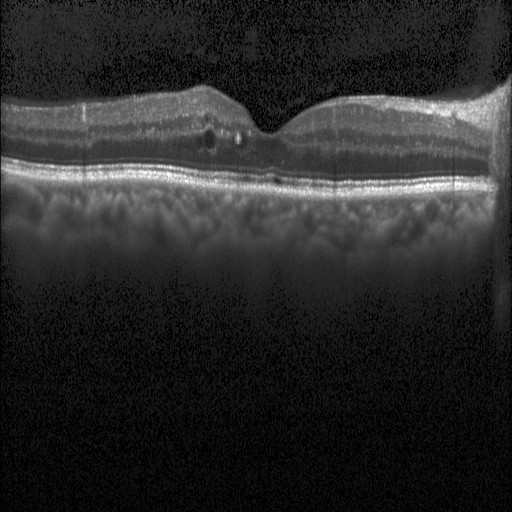

OCT B-scan showing diabetic macular edema.